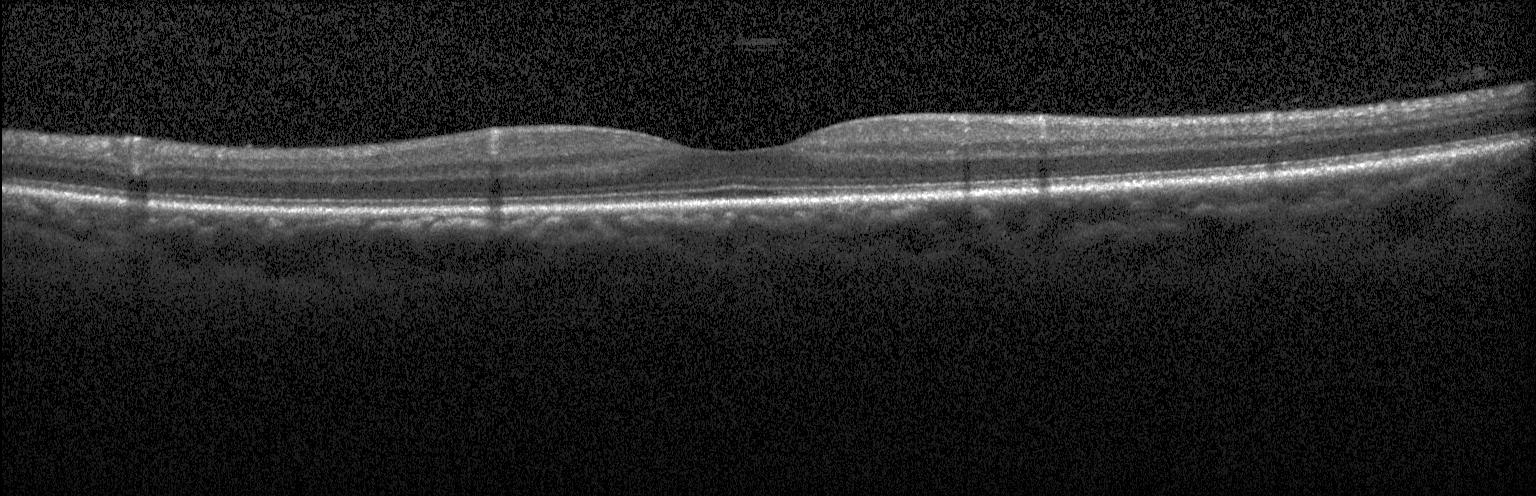

Spectral-domain OCT. Fovea-centered. Retinal OCT B-scan.
Diagnosis: no choroidal neovascularization, no diabetic macular edema, and no drusen.